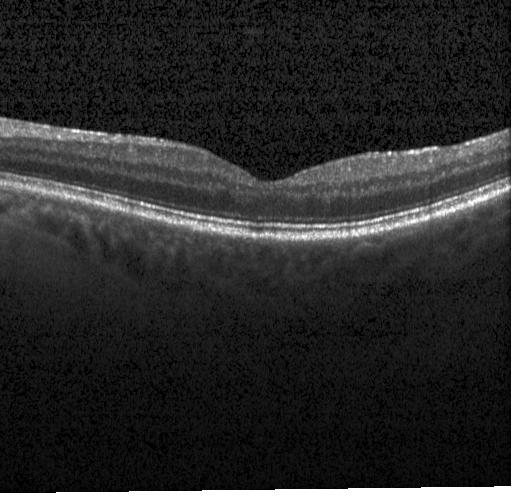

Optical coherence tomography B-scan. Through the macula — OCT finding: no CNV, no DME, and no drusen.